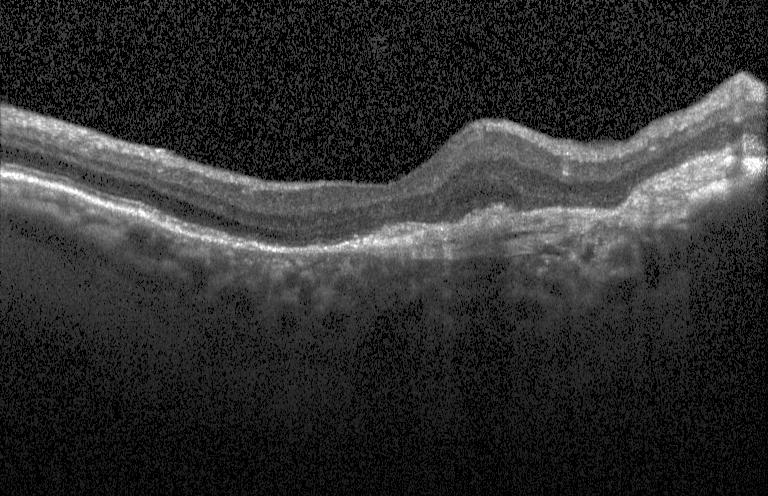

Retinal OCT B-scan · through the macula. Diagnosis: choroidal neovascularization.